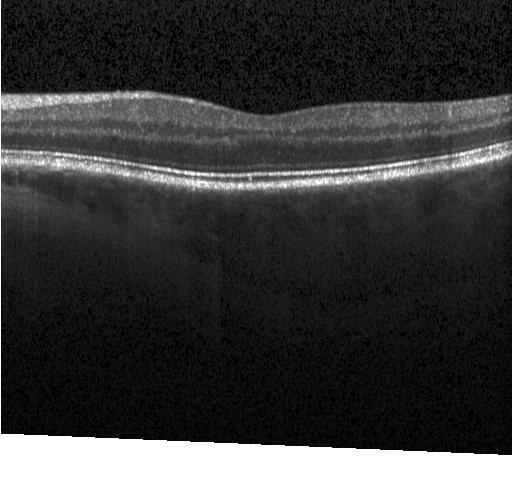

Dx: no choroidal neovascularization, diabetic macular edema, or drusen.